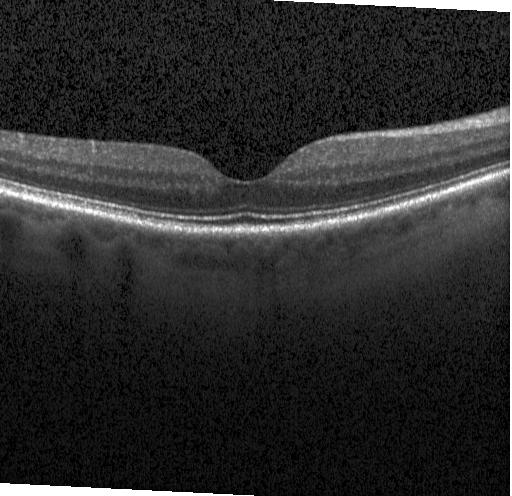
Retinal OCT cross-section showing neither CNV, DME, nor drusen.